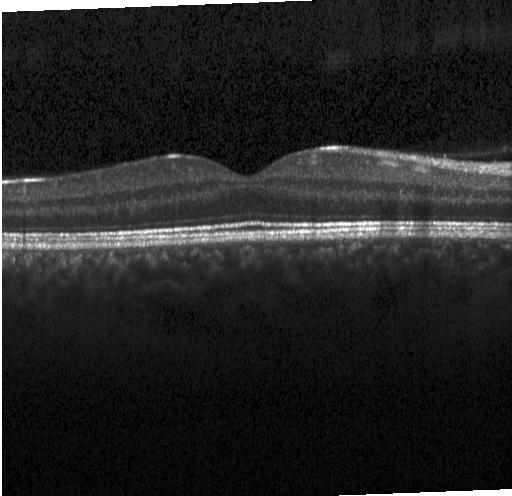 Heidelberg Spectralis OCT system; SD-OCT; OCT B-scan; through the macula.
Assessment: no choroidal neovascularization, diabetic macular edema, or drusen.